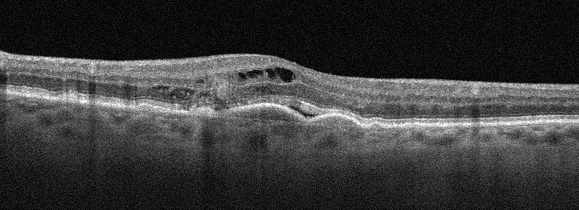

Retinal OCT B-scan; oculus sinister.
Assessment: age-related macular degeneration (AMD).